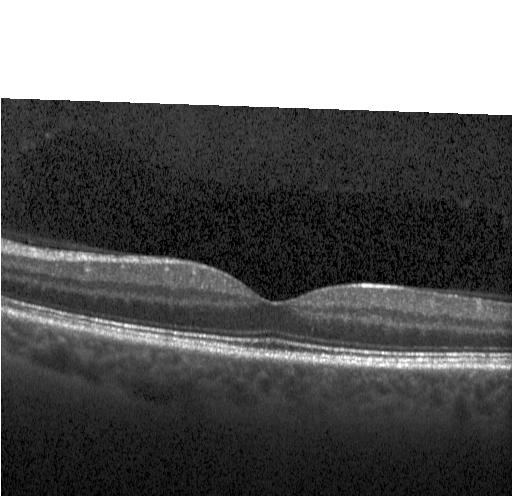
OCT line scan
The scan shows no choroidal neovascularization, no diabetic macular edema, and no drusen.